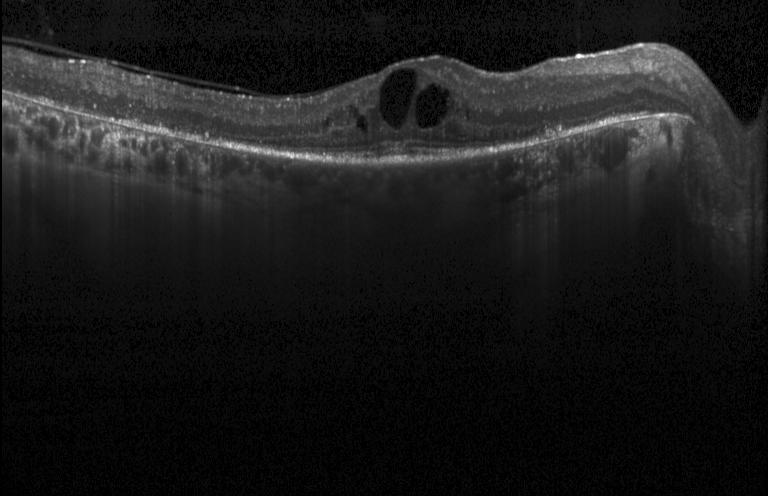 Retinal OCT cross-section. Centered on the fovea.
This B-scan demonstrates diabetic macular edema (DME).